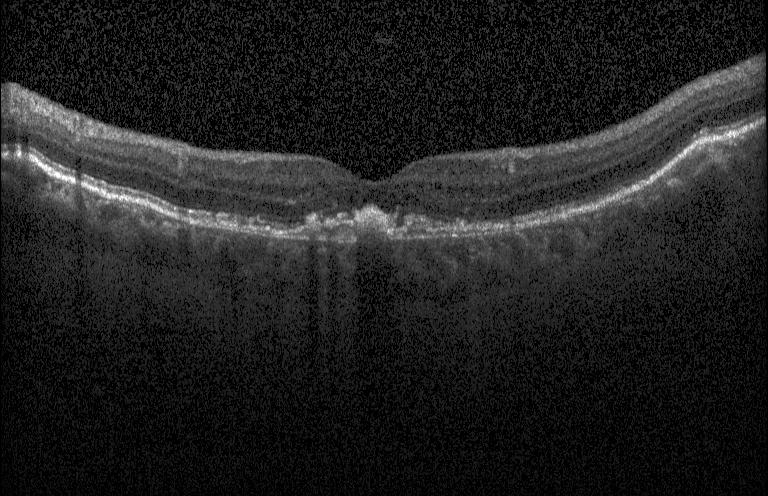

Retinal OCT B-scan. Spectral-domain optical coherence tomography. Through the macula — This B-scan demonstrates a choroidal neovascular membrane.